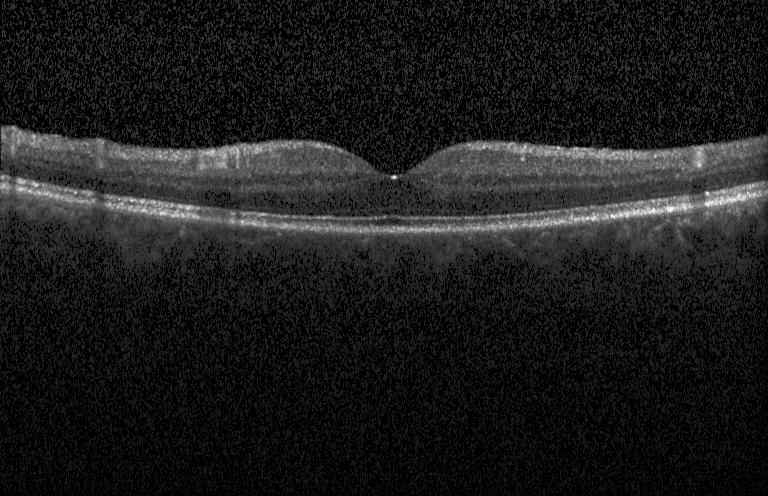 OCT line scan.
No evidence of CNV, DME, or drusen.